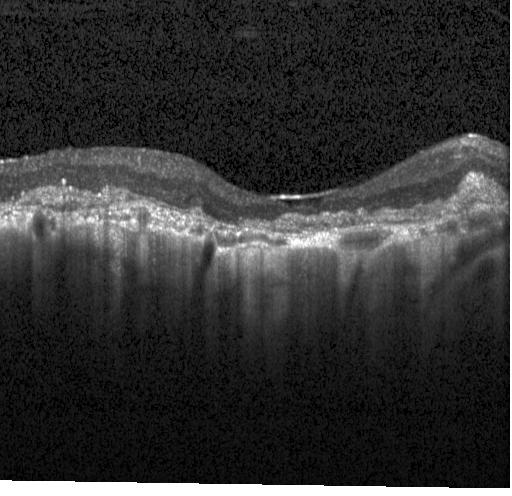
Instrument: Heidelberg Spectralis · spectral-domain optical coherence tomography · OCT B-scan.
Finding: a choroidal neovascular membrane.